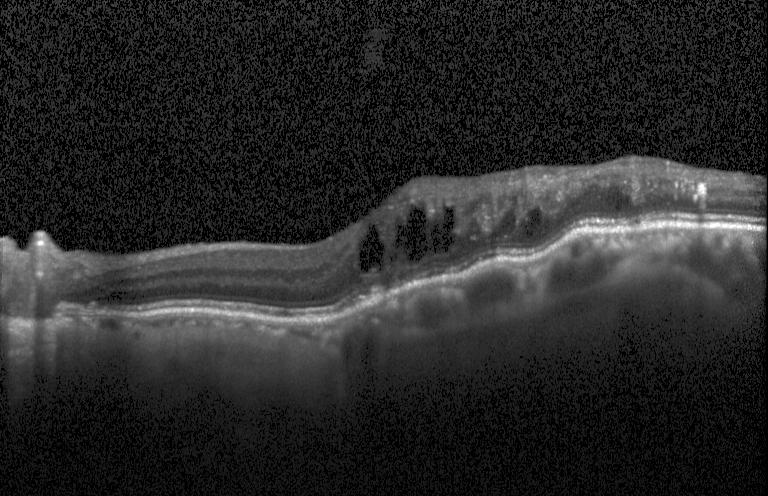

Optical coherence tomography B-scan; instrument: Heidelberg Spectralis; fovea-centered. Finding: diabetic macular edema (DME).